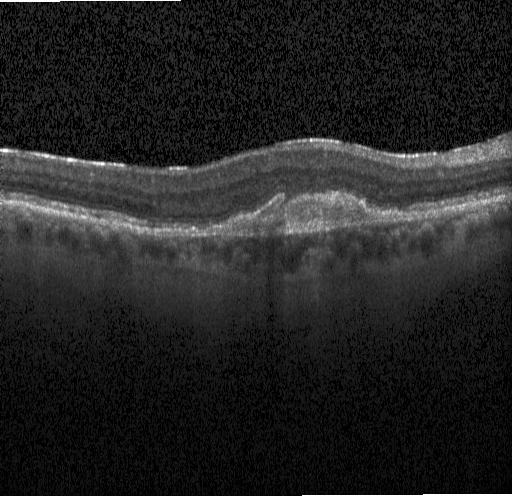
Spectral-domain optical coherence tomography; fovea-centered; OCT line scan. Assessment: a choroidal neovascular membrane.